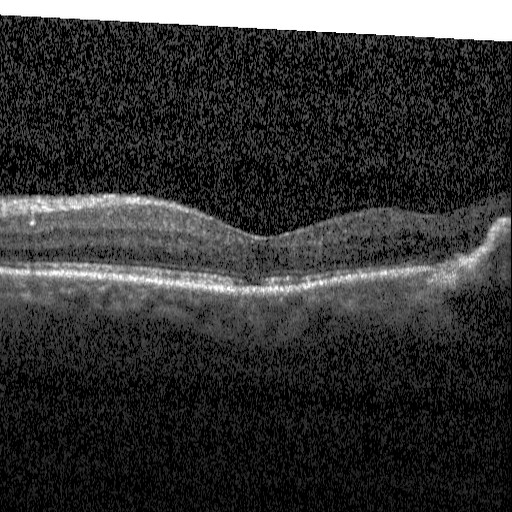

Centered on the fovea · acquired on a Heidelberg Spectralis · OCT B-scan — Impression: diabetic macular edema (DME).